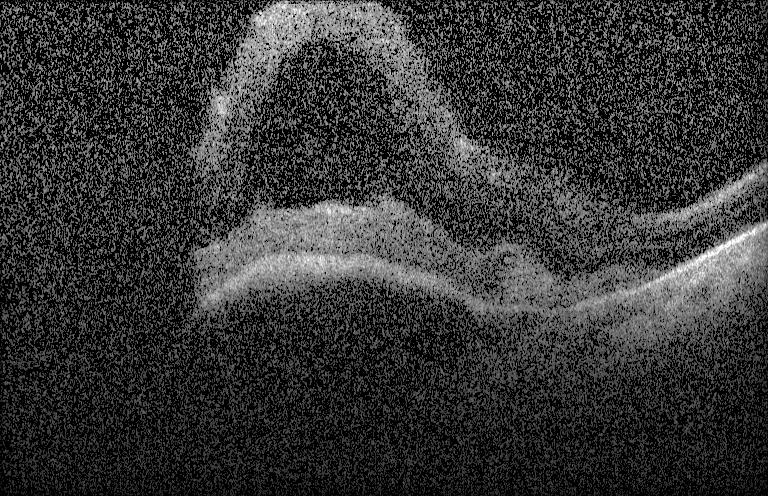 Heidelberg Spectralis OCT system; spectral-domain OCT; OCT B-scan; fovea-centered. Macular OCT: a choroidal neovascular membrane.